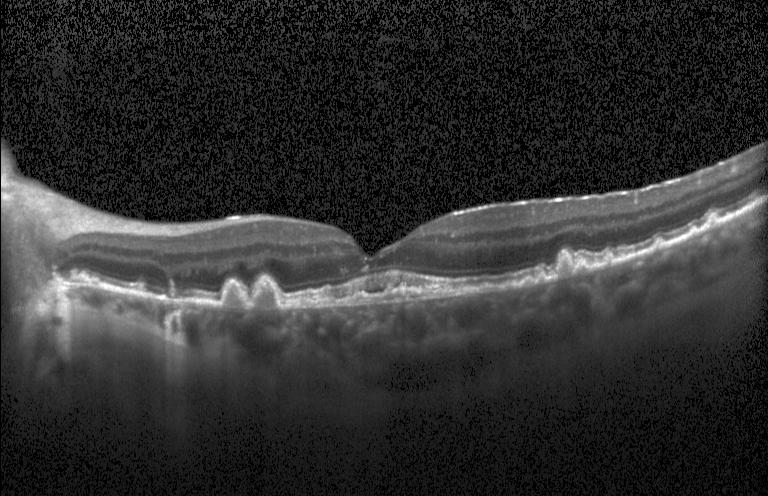 SD-OCT. Heidelberg Spectralis. Retinal OCT cross-section. Horizontal scan through the fovea — Finding: choroidal neovascularization (CNV).